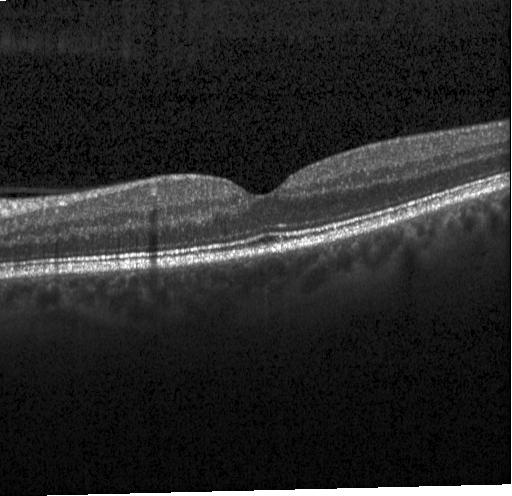
OCT B-scan. Heidelberg Spectralis. Centered on the fovea. Diagnosis: no choroidal neovascularization, diabetic macular edema, or drusen.